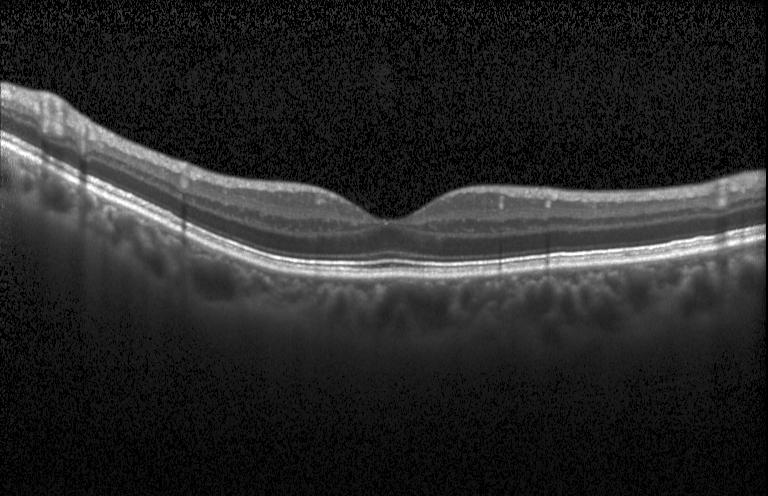
Acquired on a Heidelberg Spectralis, spectral-domain optical coherence tomography, optical coherence tomography scan
The scan shows no choroidal neovascularization, no diabetic macular edema, and no drusen.